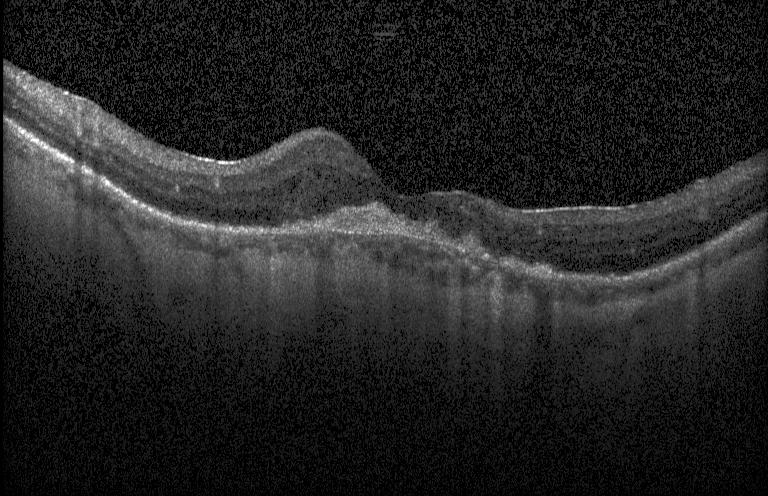 Retinal OCT cross-section showing choroidal neovascularization (CNV).